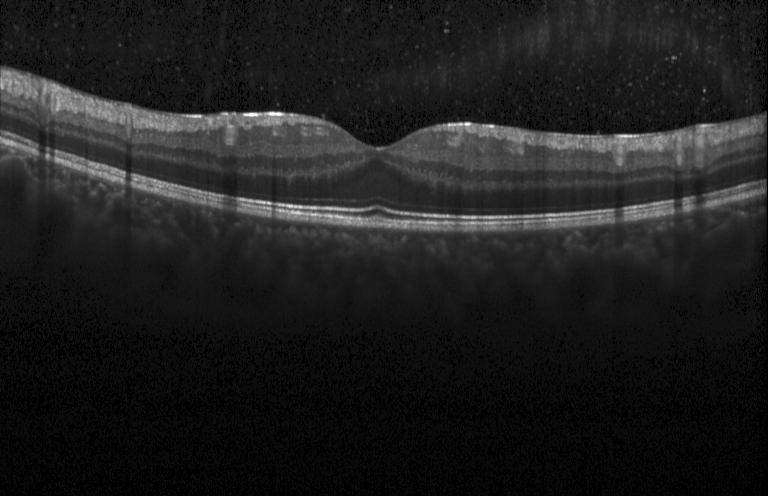
Heidelberg Spectralis · fovea-centered · spectral-domain OCT · optical coherence tomography scan.
Dx: no CNV, DME, or drusen.